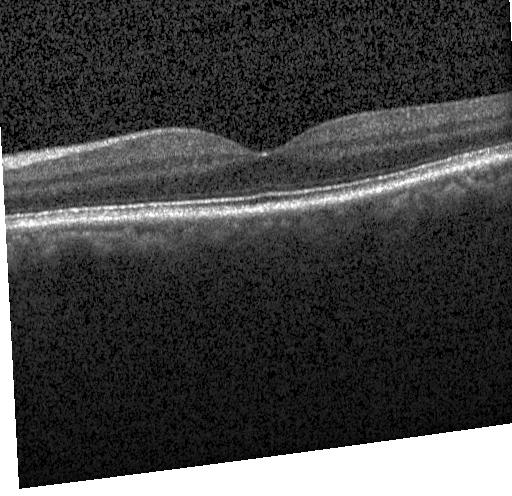

Dx: neither choroidal neovascularization, diabetic macular edema, nor drusen.